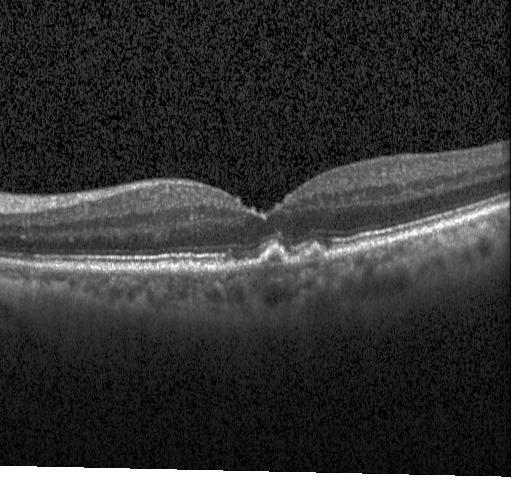 Assessment: multiple drusen.